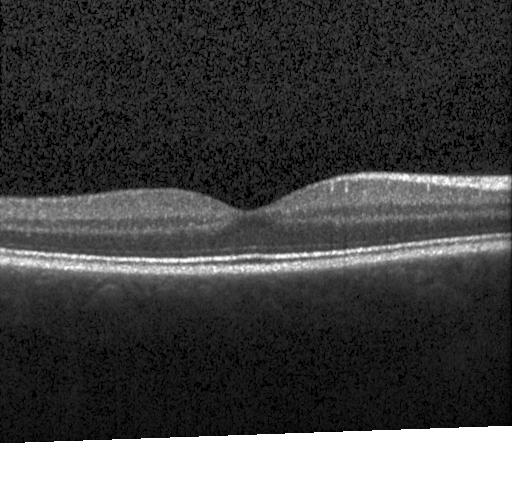

Spectral-domain OCT, acquired on a Heidelberg Spectralis, optical coherence tomography scan. The scan shows no evidence of choroidal neovascularization, diabetic macular edema, or drusen.